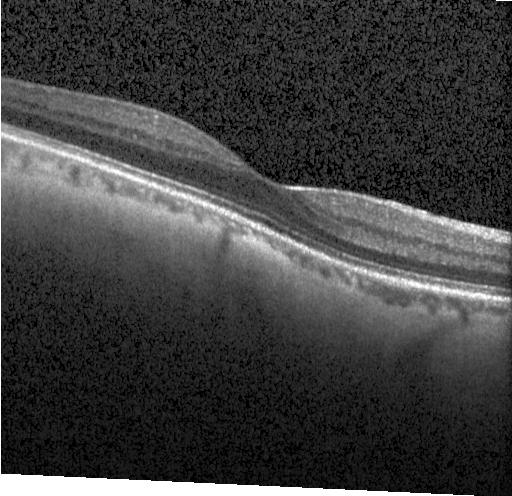

OCT line scan
Macular OCT: no choroidal neovascularization, diabetic macular edema, or drusen.